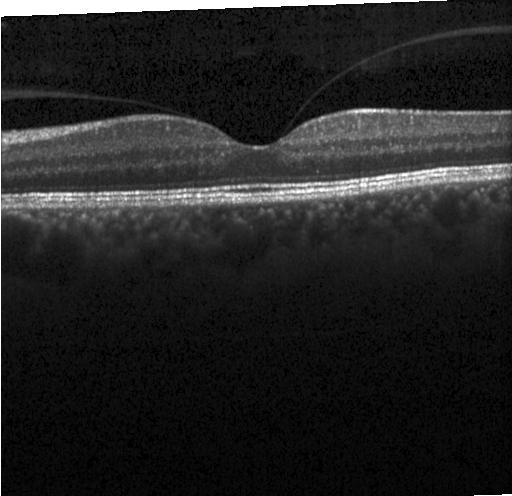 Acquired on a Heidelberg Spectralis. Macular scan. OCT line scan — Dx: neither CNV, DME, nor drusen.